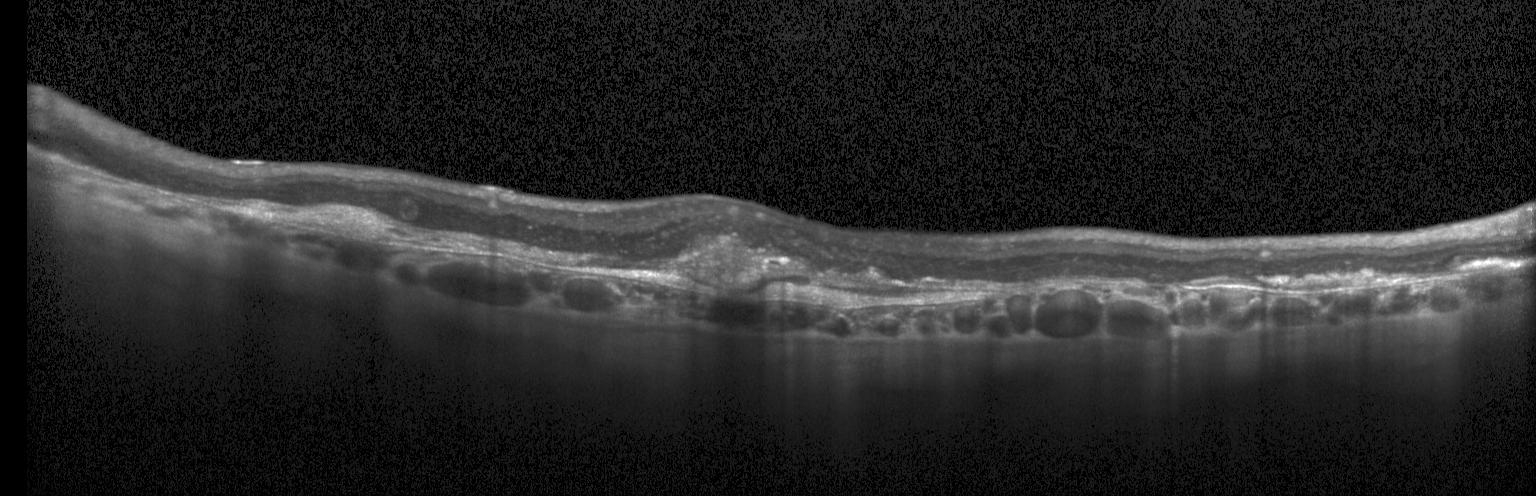 Through the macula; Heidelberg Spectralis OCT system; retinal OCT B-scan. The scan shows a choroidal neovascular membrane.